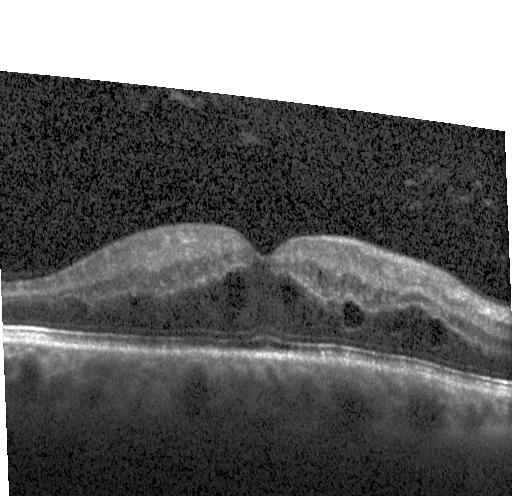 OCT B-scan.
Impression: diabetic macular edema.